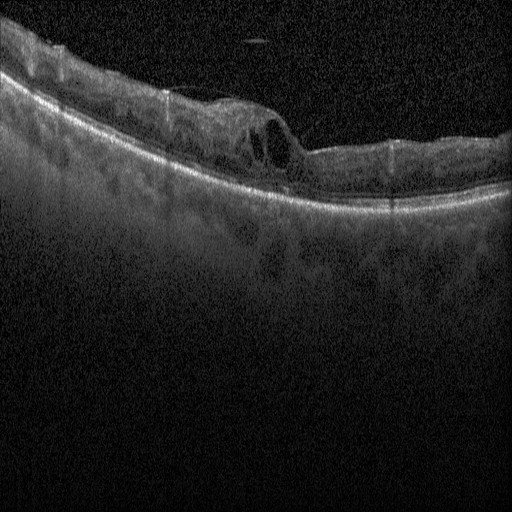 Retinal OCT cross-section · acquired on a Heidelberg Spectralis — DME.